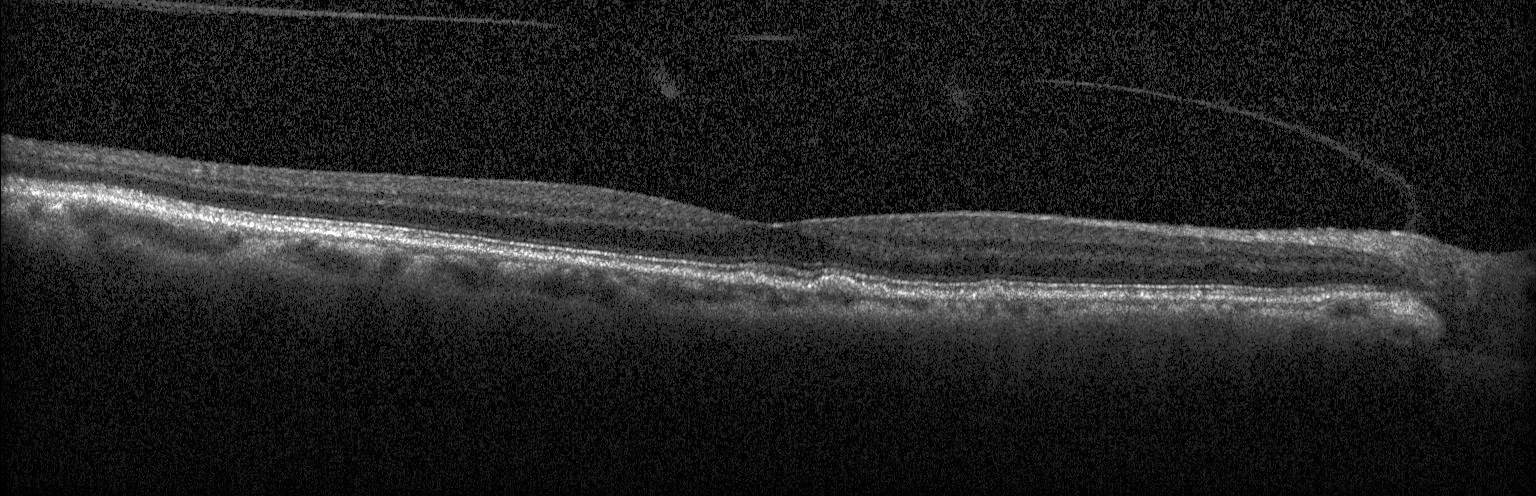 Retinal OCT B-scan · Heidelberg Spectralis · spectral-domain optical coherence tomography.
Macular OCT: sub-RPE drusenoid deposits.